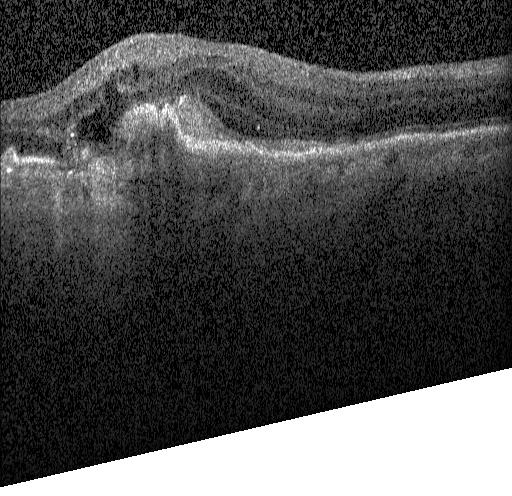

Spectral-domain OCT · instrument: Heidelberg Spectralis · fovea-centered · retinal OCT cross-section. A choroidal neovascular membrane.